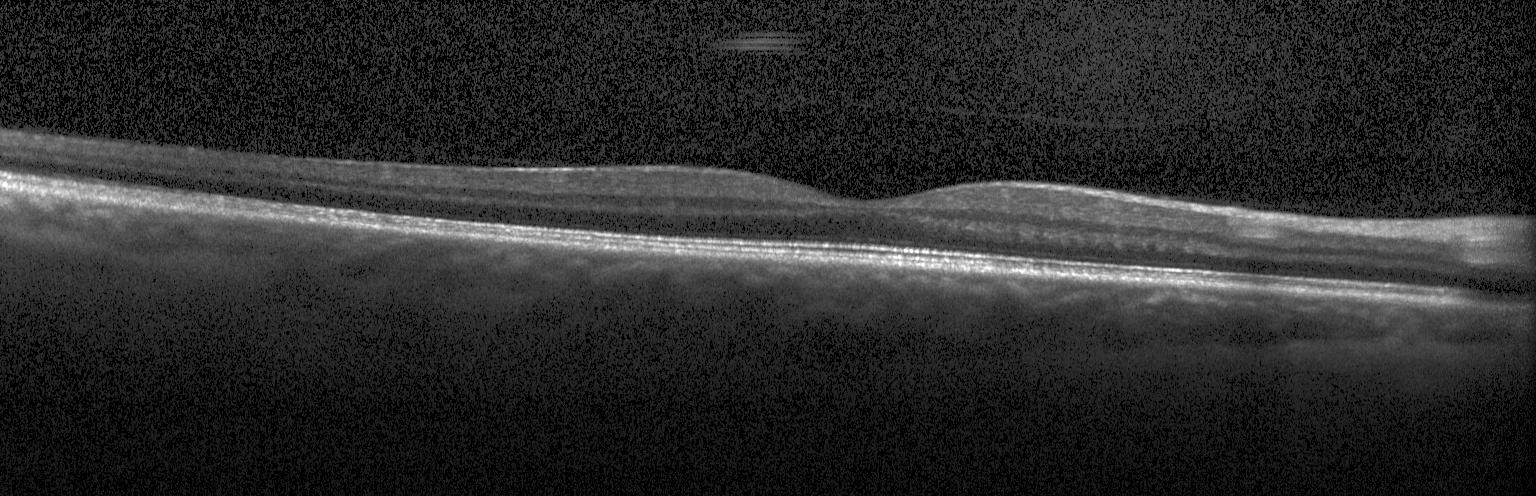
Heidelberg Spectralis; fovea-centered; spectral-domain optical coherence tomography; OCT line scan
The scan shows neither choroidal neovascularization, diabetic macular edema, nor drusen.